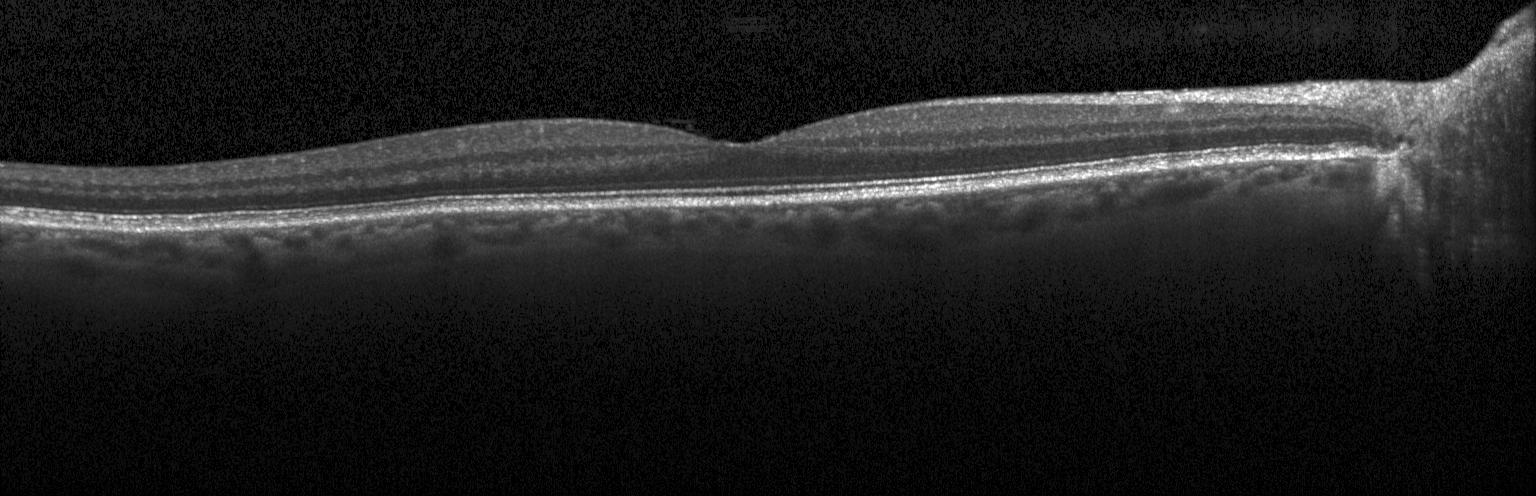 Acquired on a Heidelberg Spectralis, retinal OCT B-scan.
Assessment: neither choroidal neovascularization, diabetic macular edema, nor drusen.